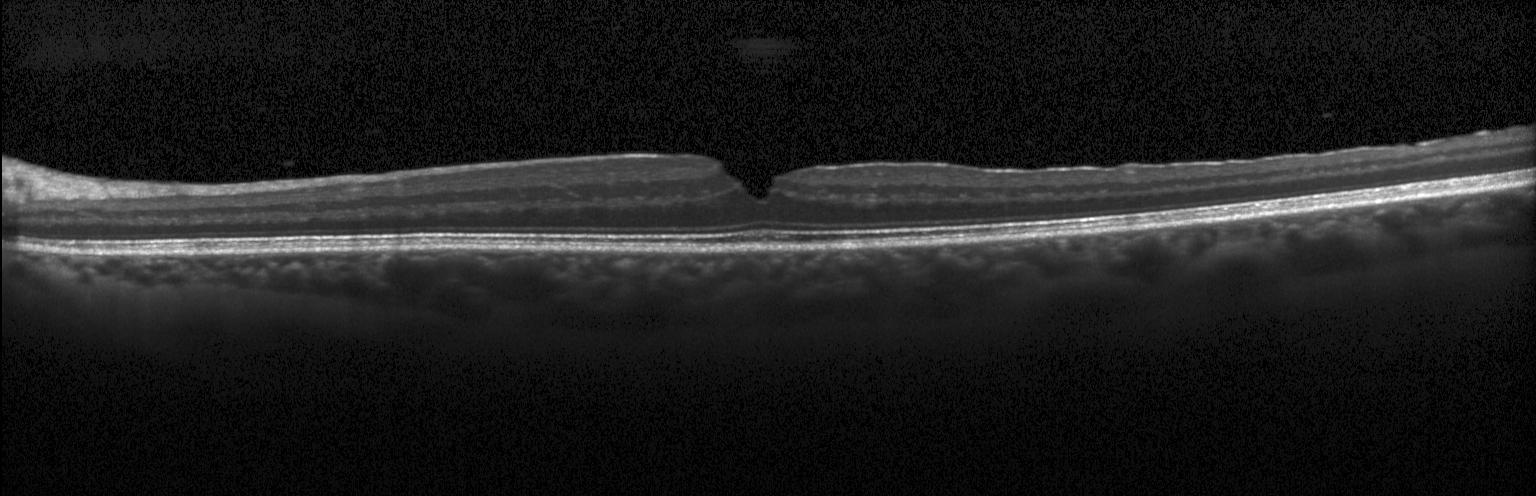

Retinal OCT cross-section; horizontal scan through the fovea — Finding: neither choroidal neovascularization, diabetic macular edema, nor drusen.